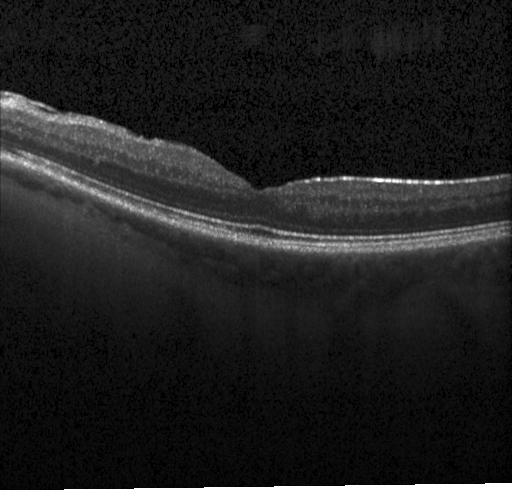

The scan shows no choroidal neovascularization, diabetic macular edema, or drusen.